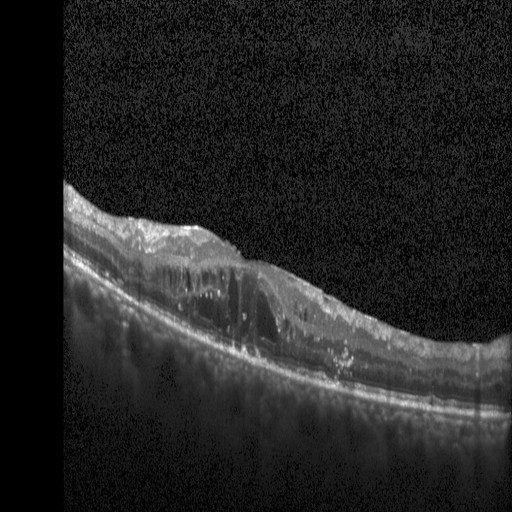

Heidelberg Spectralis; SD-OCT; centered on the fovea; optical coherence tomography scan. Diagnosis: diabetic macular edema (DME).